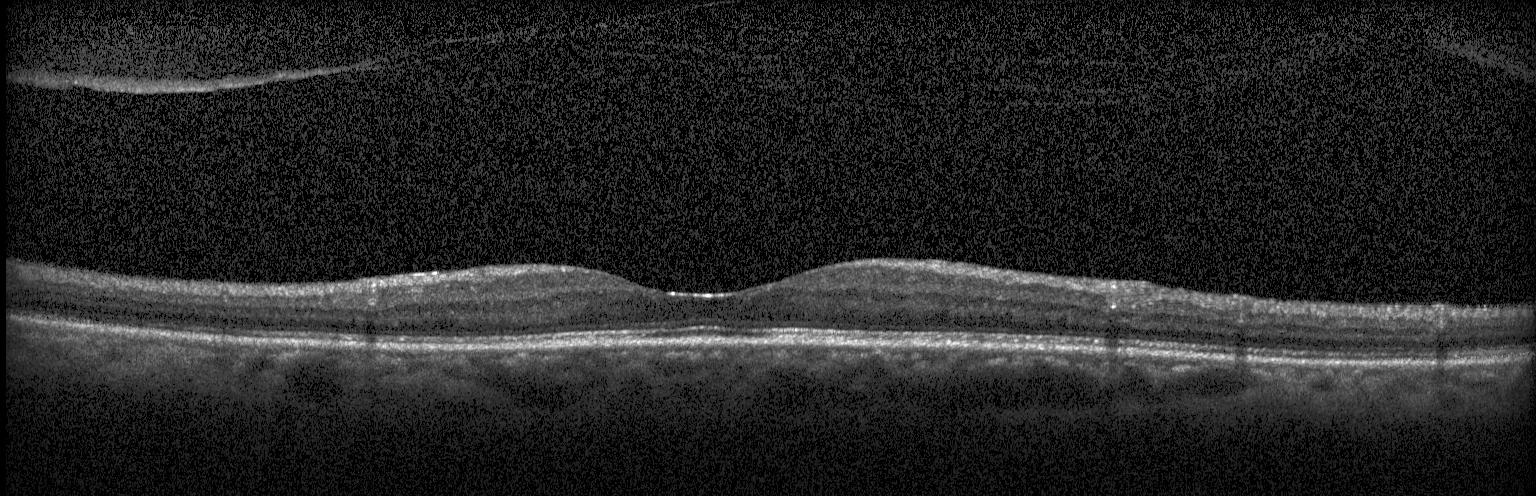 Retinal OCT cross-section showing no evidence of choroidal neovascularization, diabetic macular edema, or drusen.